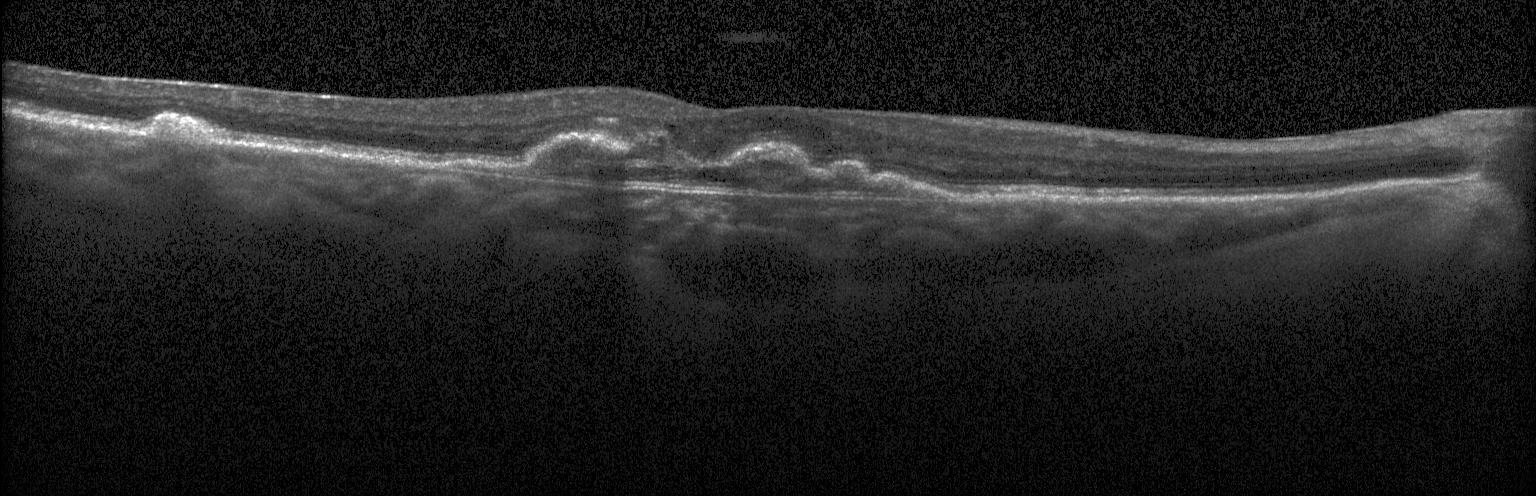 OCT finding: CNV.